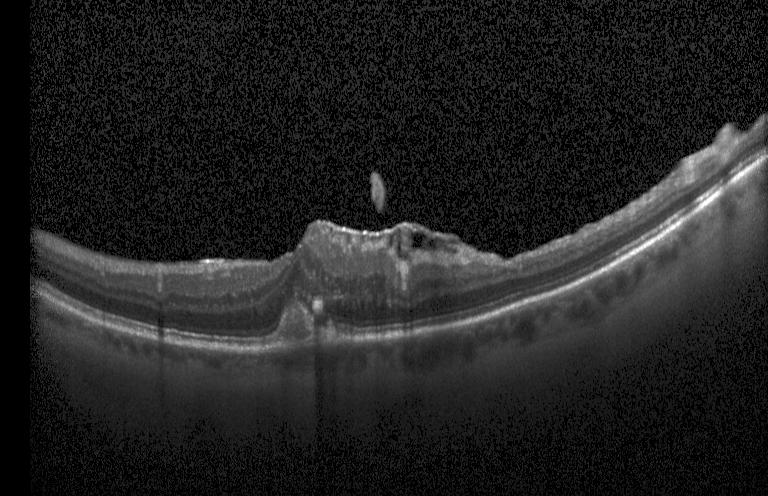
OCT line scan
Macular OCT: a choroidal neovascular membrane.